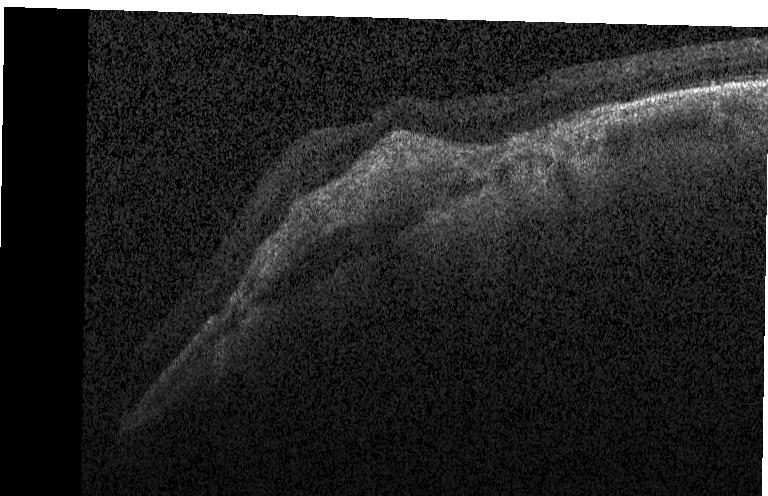 Optical coherence tomography scan. Horizontal scan through the fovea
Impression: choroidal neovascularization (CNV).